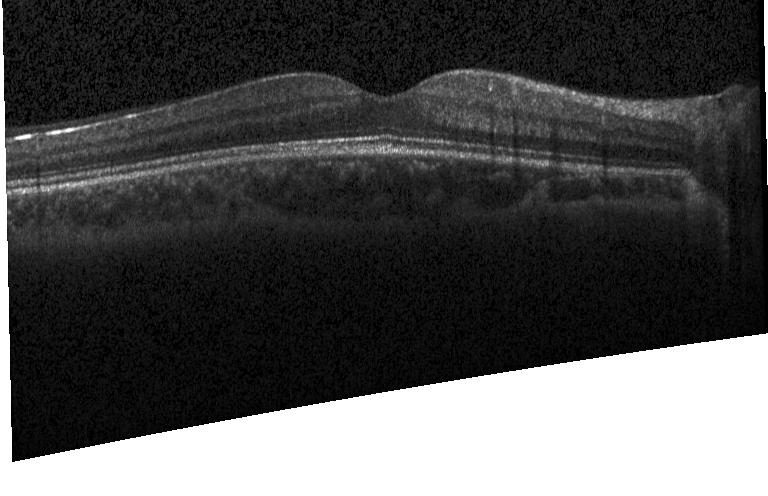

Spectral-domain OCT. Centered on the fovea. Acquired on a Heidelberg Spectralis. OCT line scan — Dx: no CNV, no DME, and no drusen.